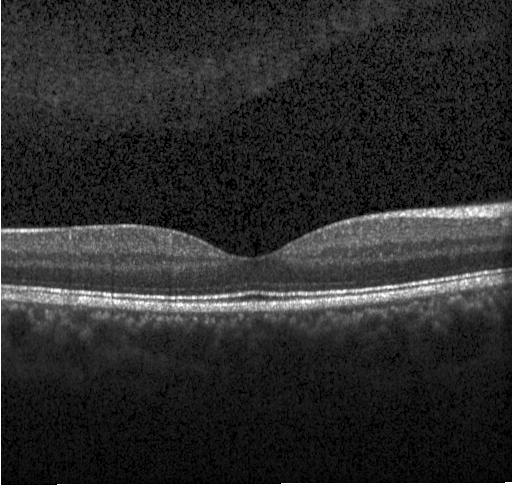
Dx: no evidence of choroidal neovascularization, diabetic macular edema, or drusen.